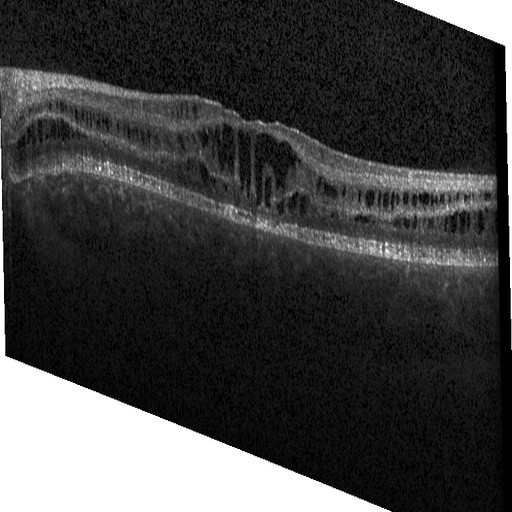 Diagnosis: diabetic macular edema.